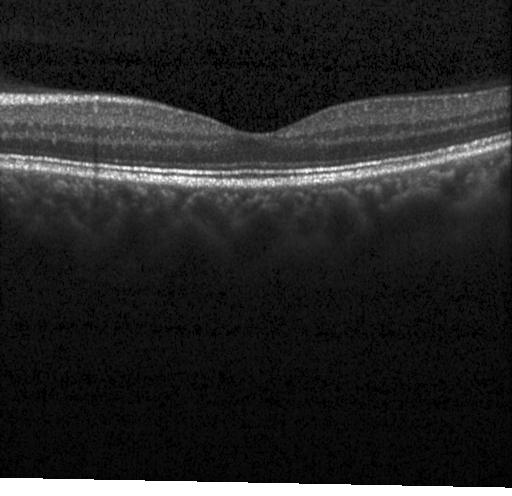
Optical coherence tomography scan; acquired on a Heidelberg Spectralis — Diagnosis: no CNV, DME, or drusen.